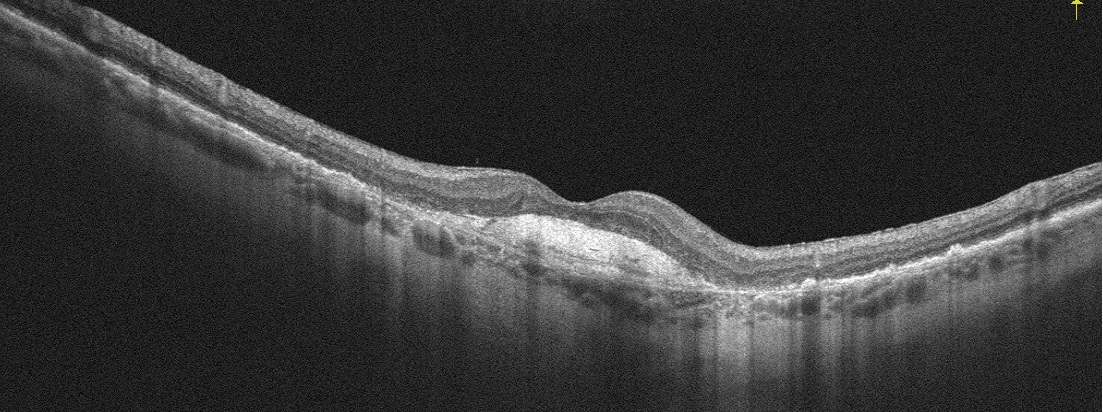

Retinal OCT B-scan — Impression: AMD.